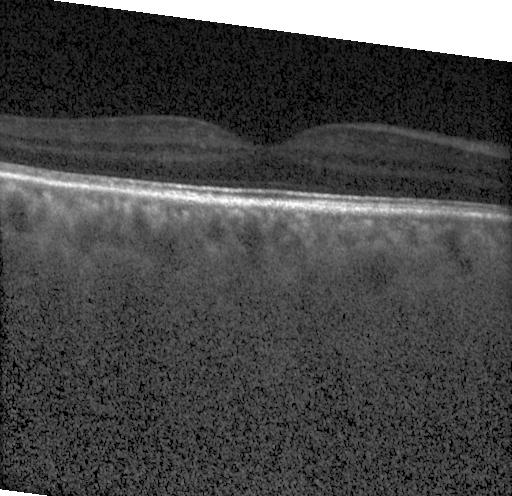

Macular OCT: neither choroidal neovascularization, diabetic macular edema, nor drusen.